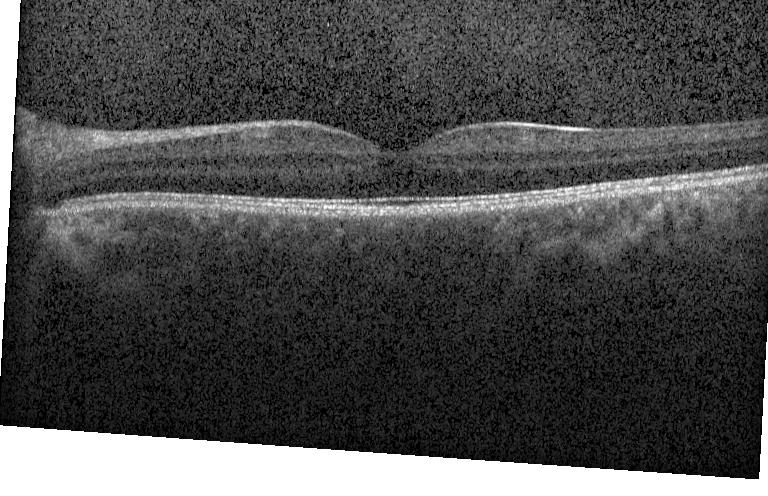 OCT B-scan — Diagnosis: no choroidal neovascularization, diabetic macular edema, or drusen.